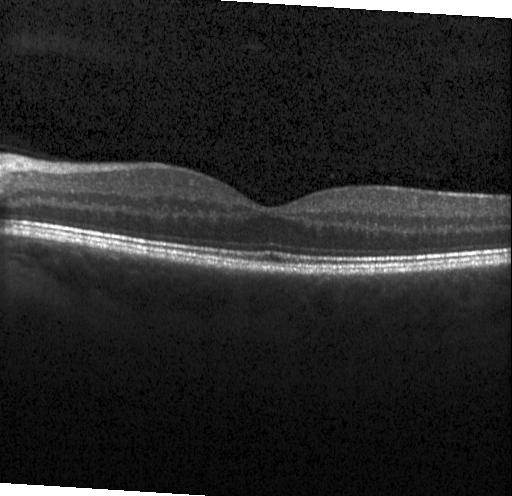 Spectral-domain OCT · OCT B-scan · acquired on a Heidelberg Spectralis. Impression: no CNV, no DME, and no drusen.